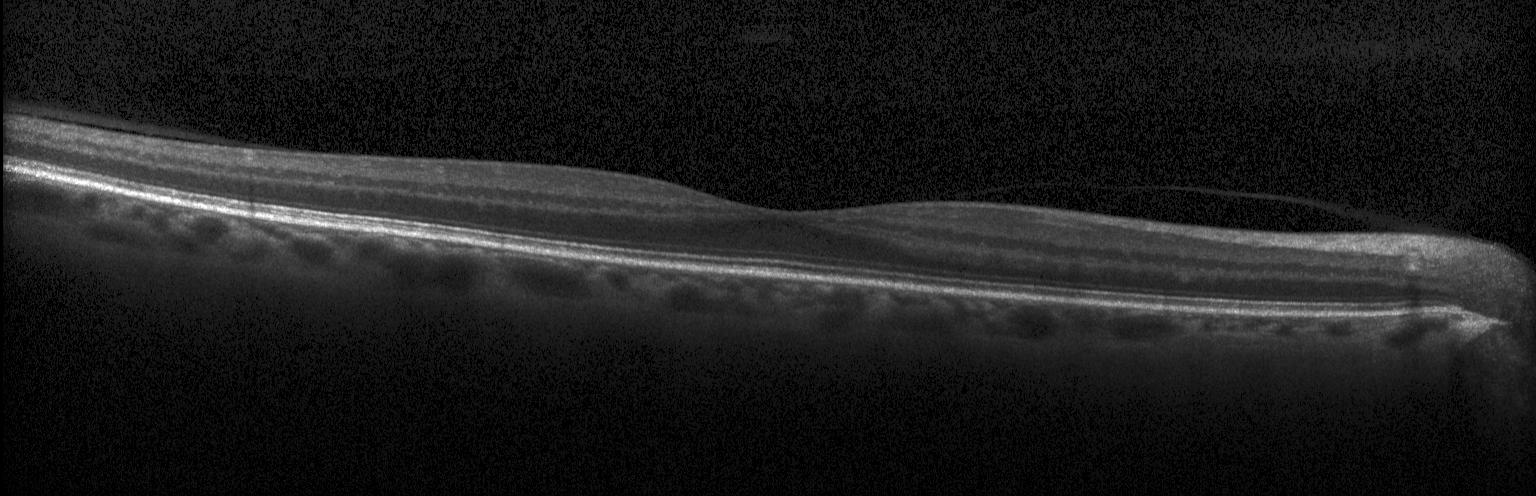 Impression: neither choroidal neovascularization, diabetic macular edema, nor drusen.